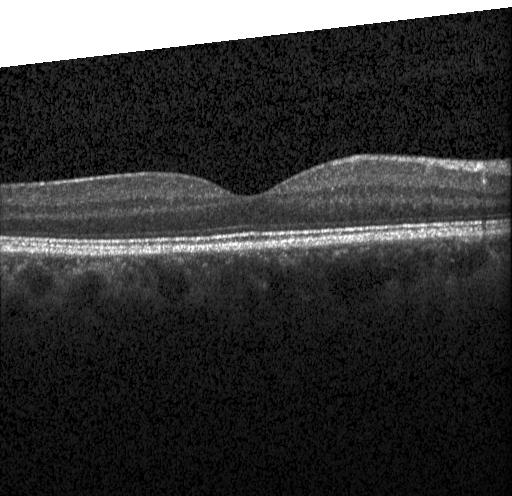
OCT B-scan showing no CNV, DME, or drusen.